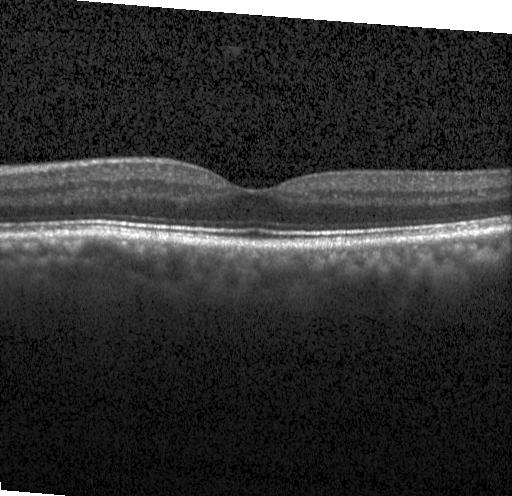 Spectral-domain OCT · acquired on a Heidelberg Spectralis · optical coherence tomography B-scan · horizontal scan through the fovea.
Impression: no choroidal neovascularization, no diabetic macular edema, and no drusen.